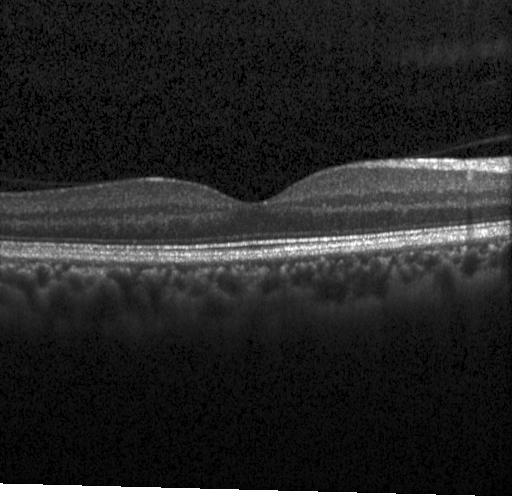
This B-scan demonstrates neither choroidal neovascularization, diabetic macular edema, nor drusen.